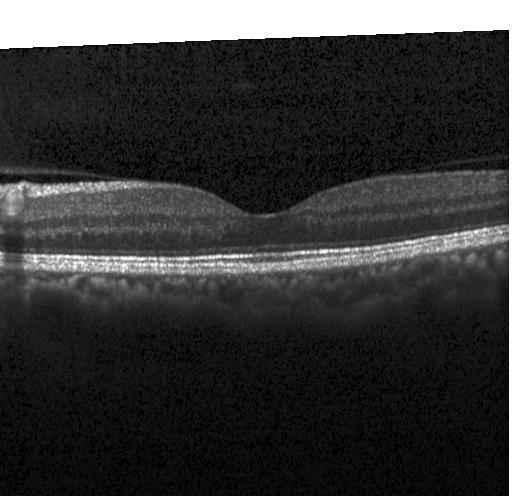

Through the macula, optical coherence tomography B-scan, SD-OCT — Diagnosis: no evidence of CNV, DME, or drusen.